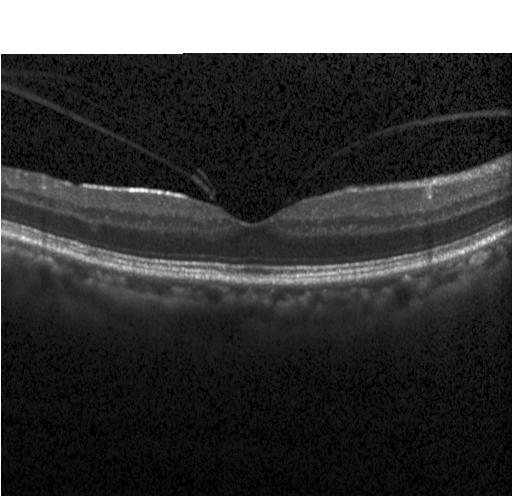
Impression: no choroidal neovascularization, no diabetic macular edema, and no drusen.